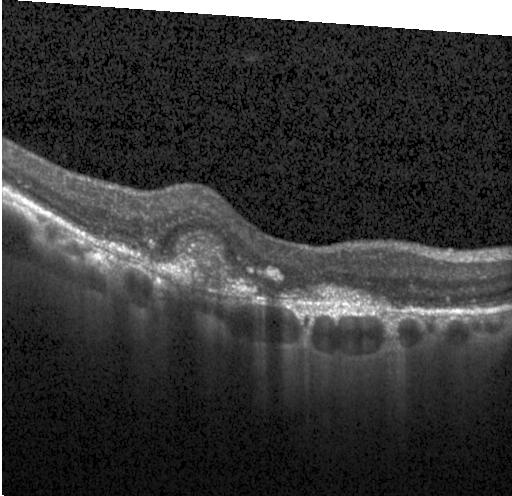 Macular scan · acquired on a Heidelberg Spectralis · OCT B-scan — Impression: a choroidal neovascular membrane.